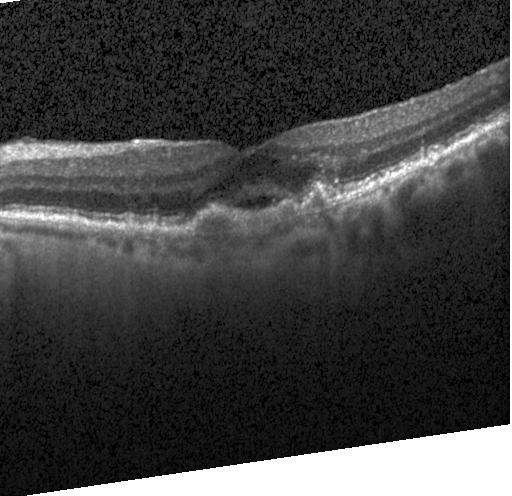
Diagnosis: choroidal neovascularization (CNV).